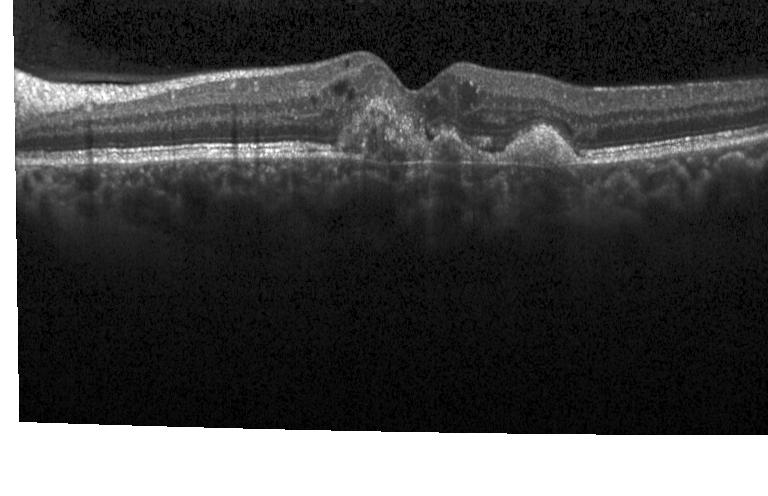
Acquired on a Heidelberg Spectralis, optical coherence tomography B-scan.
The scan shows a choroidal neovascular membrane.